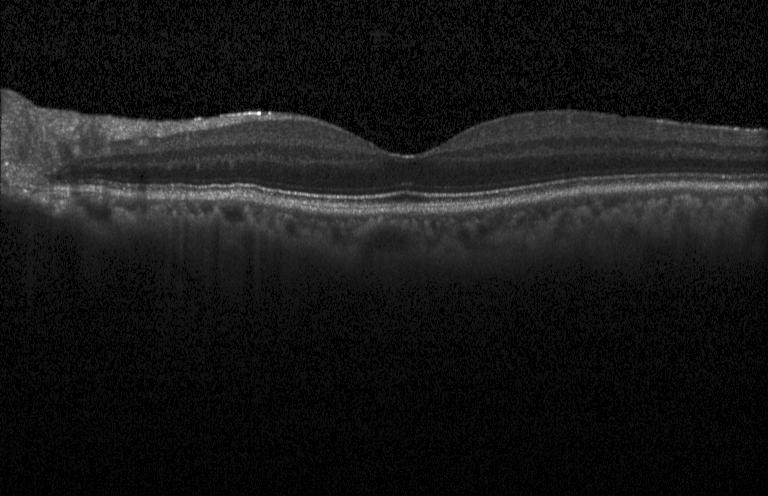

Heidelberg Spectralis OCT system, SD-OCT, optical coherence tomography scan.
The scan shows no choroidal neovascularization, no diabetic macular edema, and no drusen.